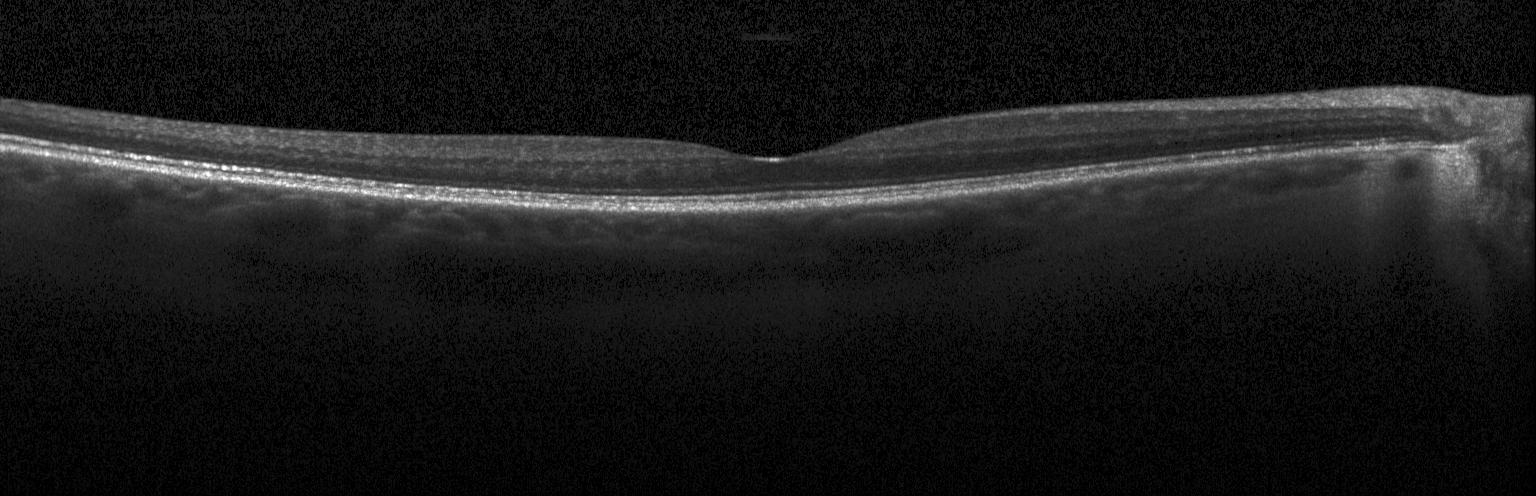

Finding: no choroidal neovascularization, diabetic macular edema, or drusen.